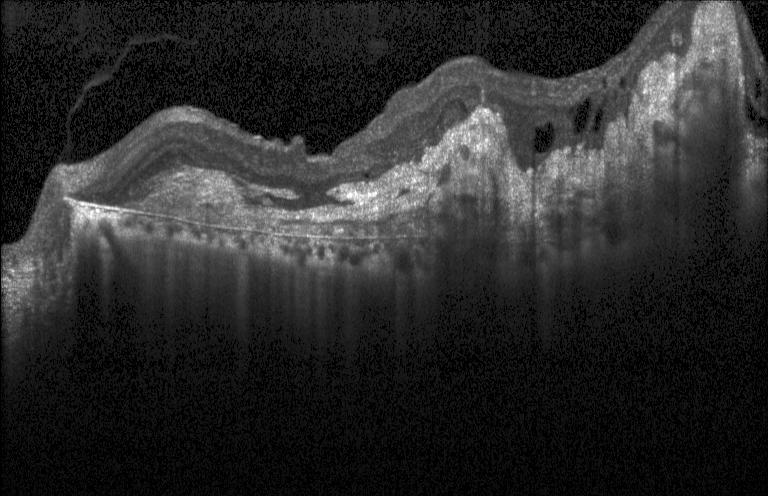 Spectral-domain OCT, OCT B-scan, through the macula, acquired on a Heidelberg Spectralis.
Diagnosis: a choroidal neovascular membrane.